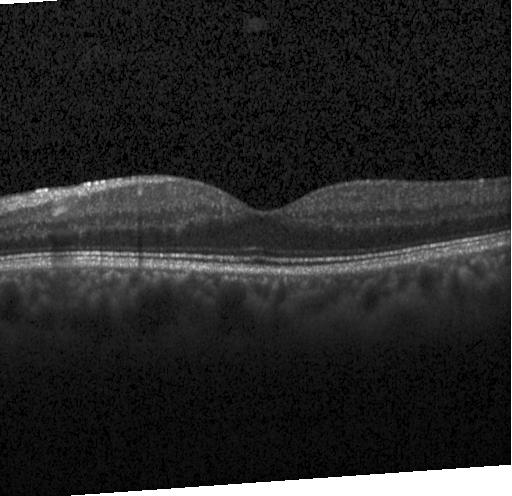

OCT B-scan. Diagnosis: no evidence of choroidal neovascularization, diabetic macular edema, or drusen.